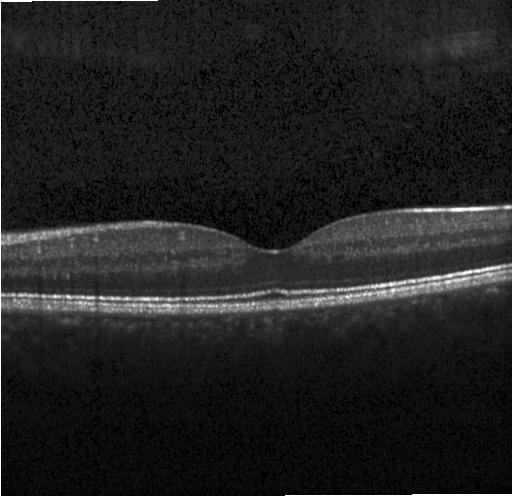
Heidelberg Spectralis · macular scan · optical coherence tomography scan.
Finding: no evidence of choroidal neovascularization, diabetic macular edema, or drusen.